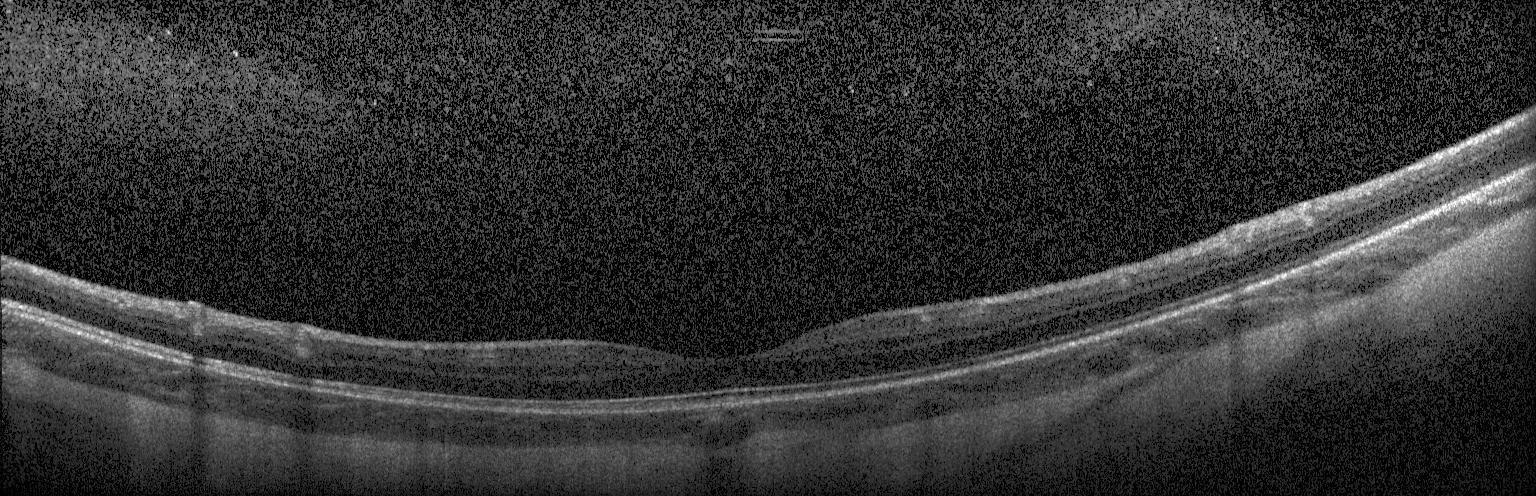

Retinal OCT B-scan · Heidelberg Spectralis.
The scan shows no evidence of choroidal neovascularization, diabetic macular edema, or drusen.